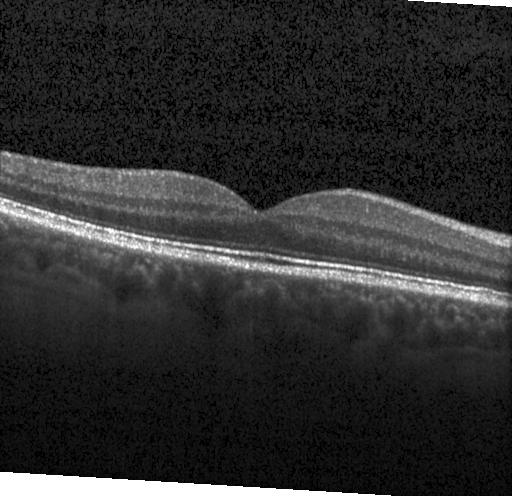 Impression: no choroidal neovascularization, no diabetic macular edema, and no drusen.